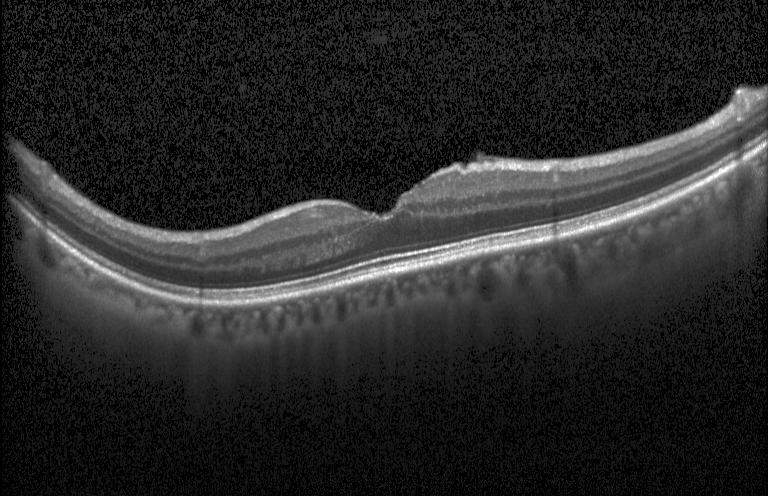 Retinal OCT B-scan; SD-OCT.
Finding: neither CNV, DME, nor drusen.